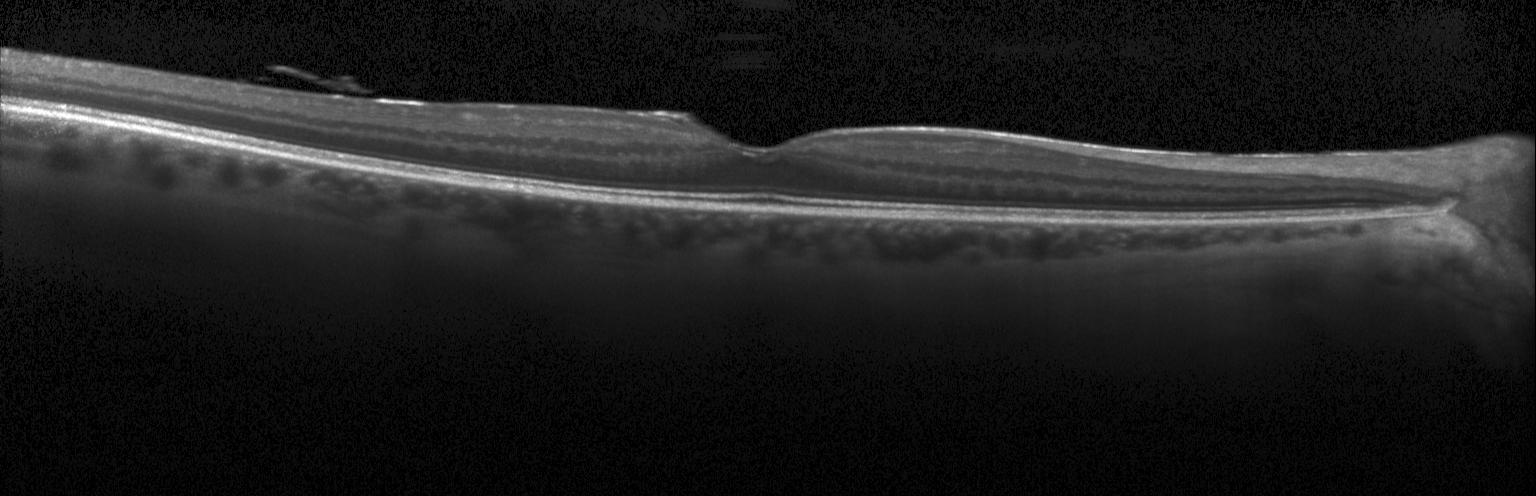
Instrument: Heidelberg Spectralis · OCT line scan · fovea-centered.
Neither choroidal neovascularization, diabetic macular edema, nor drusen.